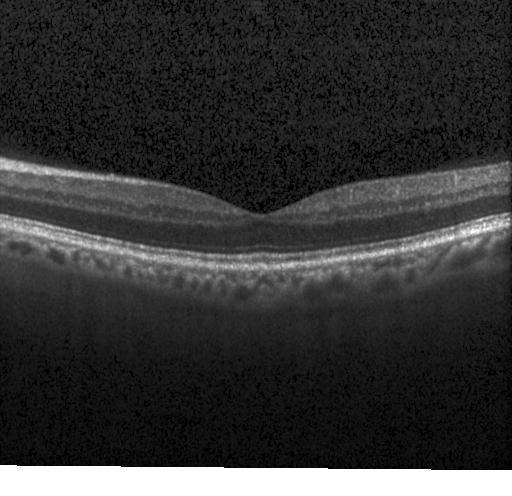
Optical coherence tomography B-scan · SD-OCT · acquired on a Heidelberg Spectralis.
No choroidal neovascularization, diabetic macular edema, or drusen.